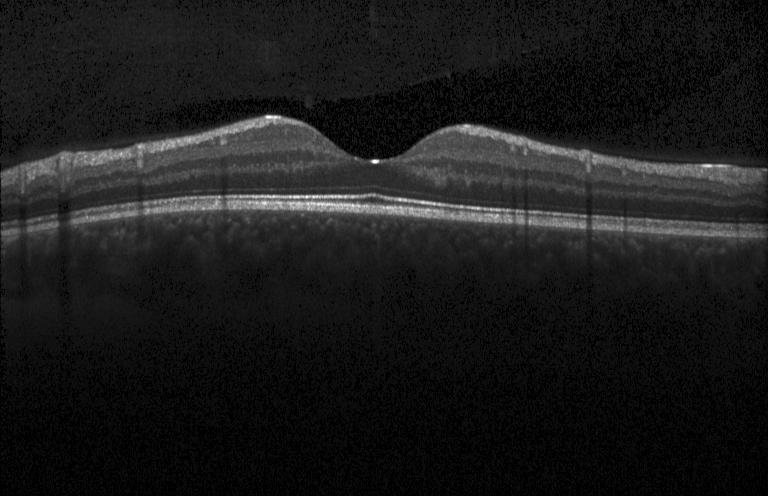

The scan shows no choroidal neovascularization, no diabetic macular edema, and no drusen.